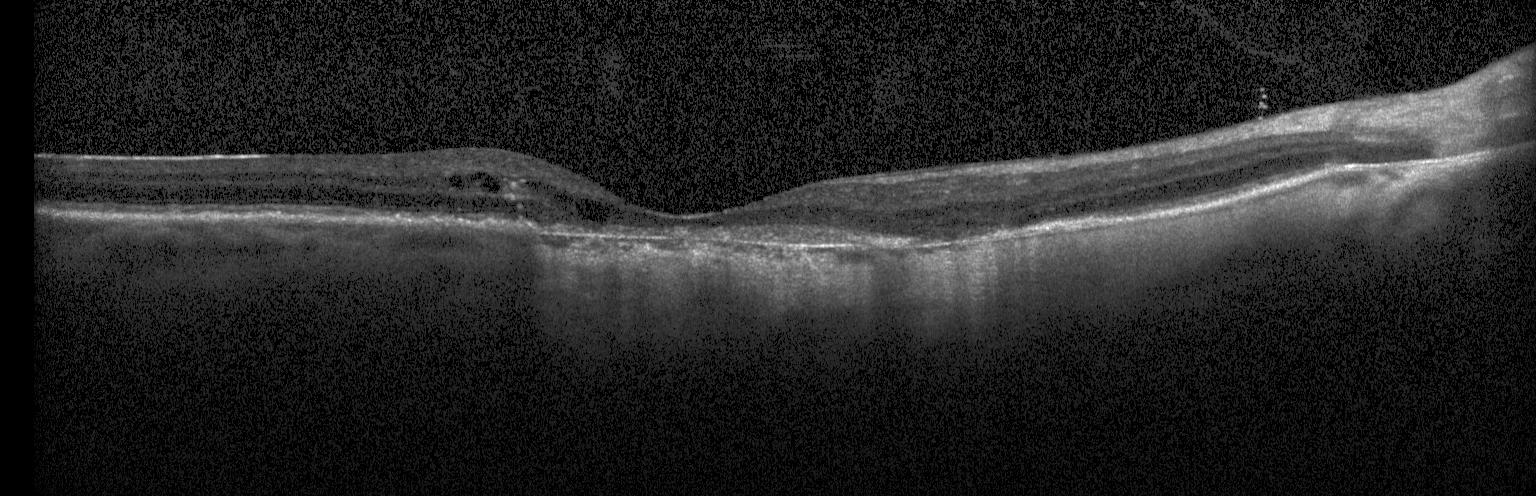 OCT B-scan, through the macula, SD-OCT, Heidelberg Spectralis.
Impression: a choroidal neovascular membrane.